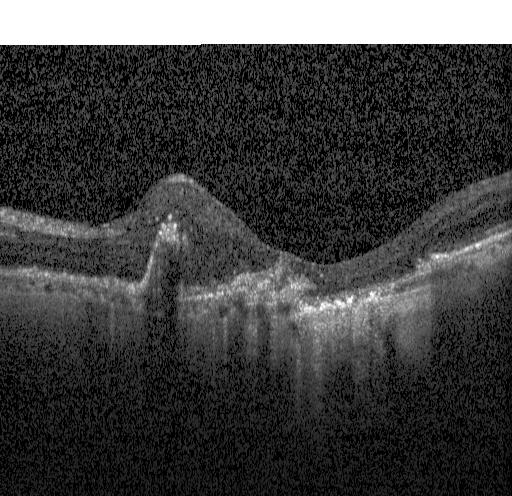
Macular OCT demonstrating choroidal neovascularization (CNV).